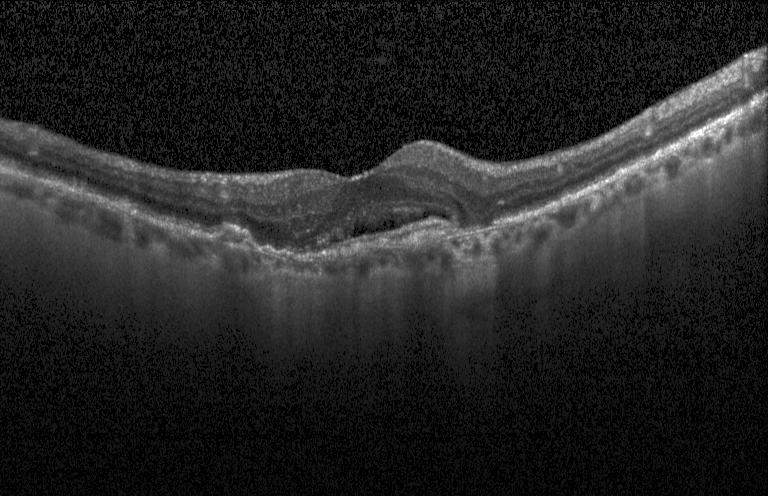

Optical coherence tomography scan · acquired on a Heidelberg Spectralis.
OCT finding: a choroidal neovascular membrane.